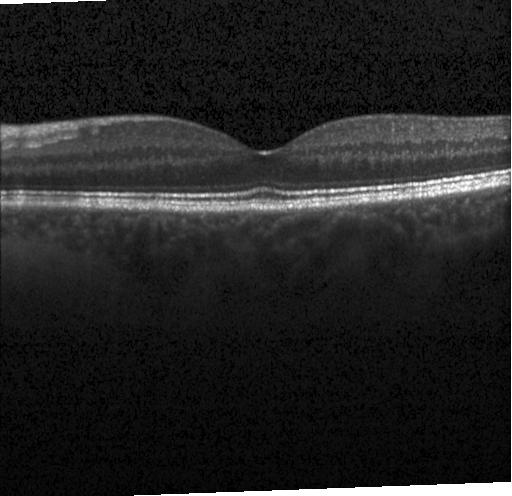 Instrument: Heidelberg Spectralis. Fovea-centered. SD-OCT. Optical coherence tomography B-scan — This B-scan demonstrates neither choroidal neovascularization, diabetic macular edema, nor drusen.